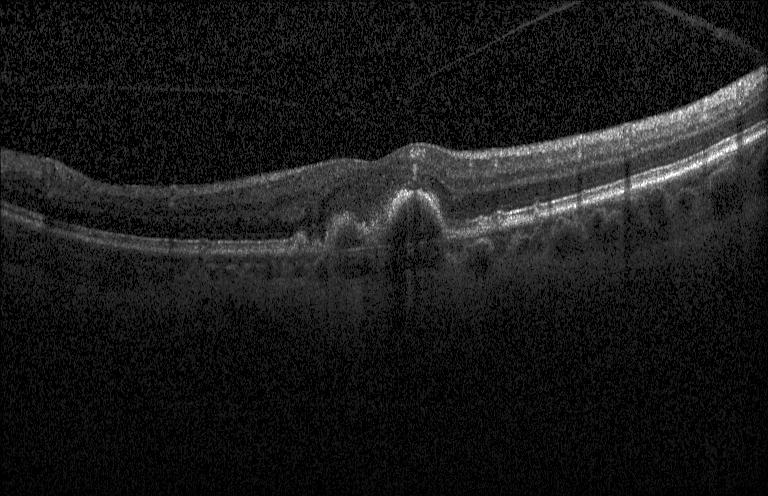
OCT finding: CNV.